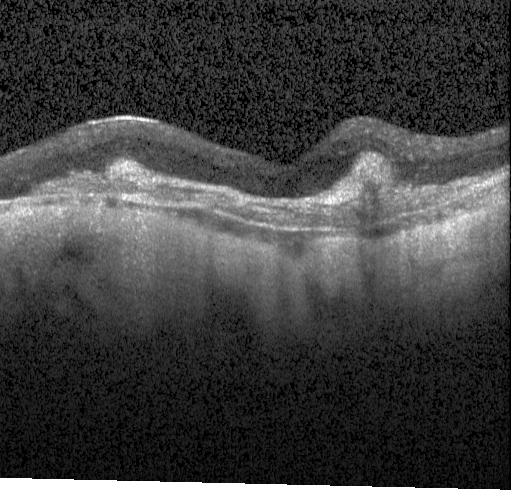
Impression: a choroidal neovascular membrane.